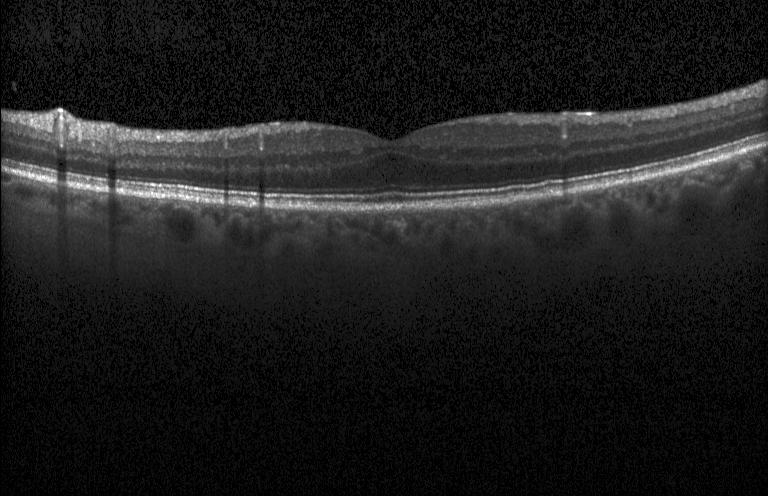
No evidence of choroidal neovascularization, diabetic macular edema, or drusen.